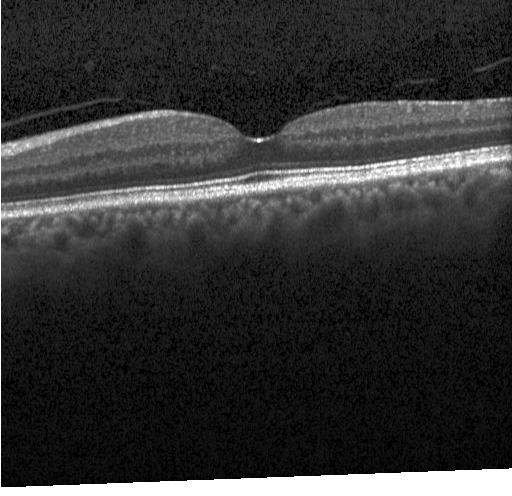

OCT line scan.
This B-scan demonstrates no choroidal neovascularization, no diabetic macular edema, and no drusen.